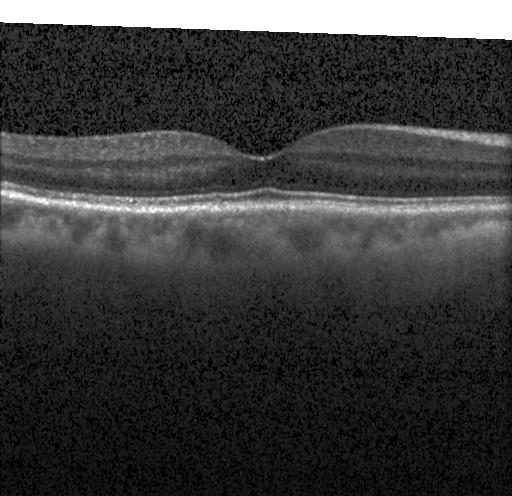

Retinal OCT B-scan · SD-OCT · Heidelberg Spectralis · centered on the fovea. OCT finding: no choroidal neovascularization, diabetic macular edema, or drusen.